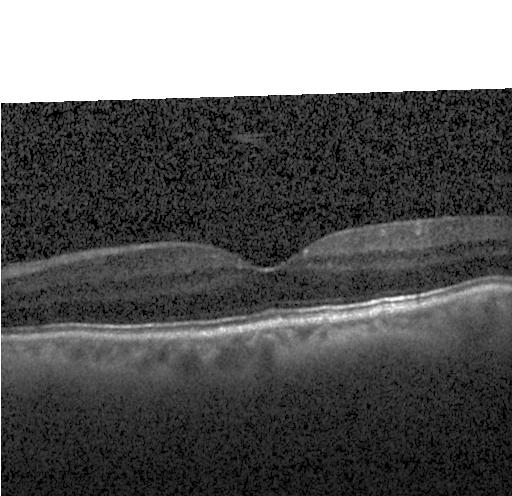
Retinal OCT B-scan; centered on the fovea
Diagnosis: no choroidal neovascularization, diabetic macular edema, or drusen.